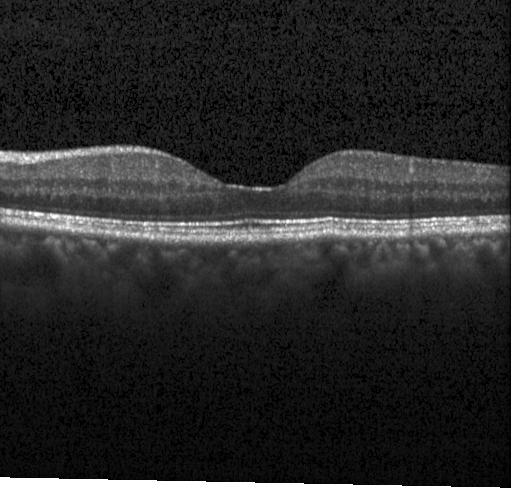 Heidelberg Spectralis OCT system; retinal OCT B-scan; spectral-domain OCT — Macular OCT: neither choroidal neovascularization, diabetic macular edema, nor drusen.